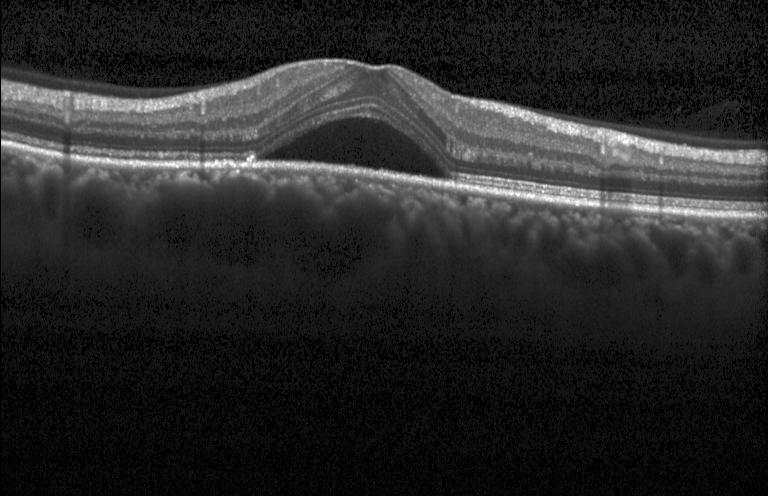

Retinal OCT cross-section; acquired on a Heidelberg Spectralis. The scan shows choroidal neovascularization.